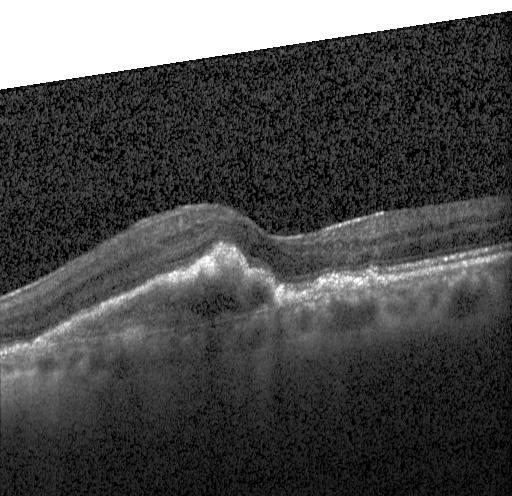
OCT B-scan, instrument: Heidelberg Spectralis.
Impression: a choroidal neovascular membrane.